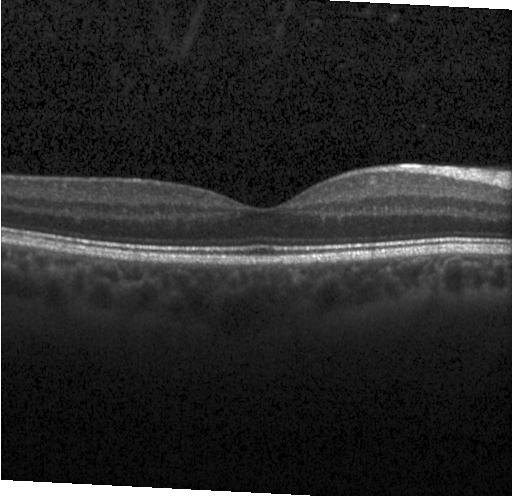 Diagnosis: no CNV, no DME, and no drusen.